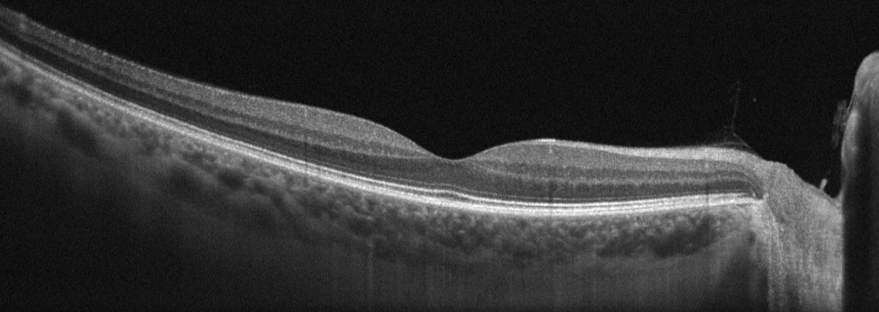
Dx: absence of AMD, DME, ERM, RAO, RVO, and vitreomacular interface disease.